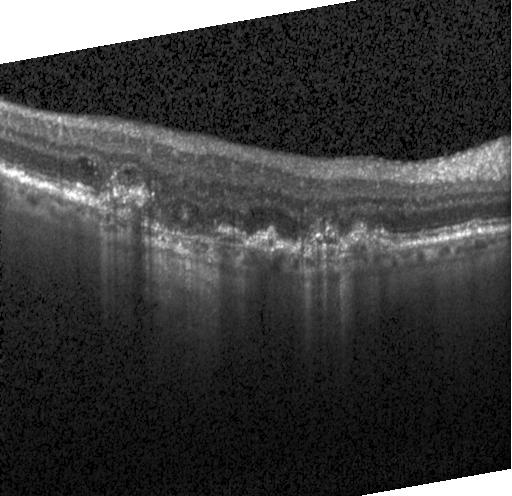

Optical coherence tomography B-scan. Heidelberg Spectralis OCT system — Dx: choroidal neovascularization (CNV).